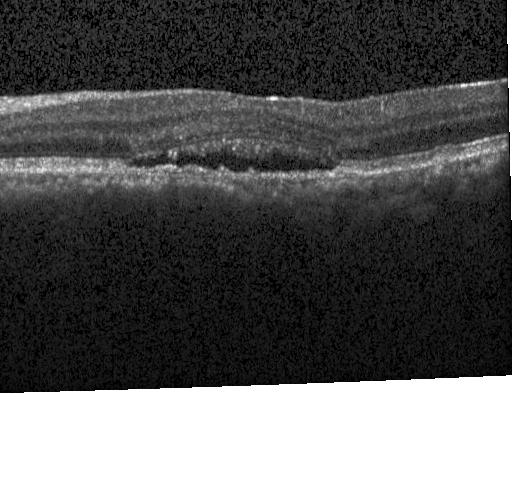

Heidelberg Spectralis OCT system · optical coherence tomography B-scan · spectral-domain optical coherence tomography · fovea-centered. Dx: choroidal neovascularization (CNV).